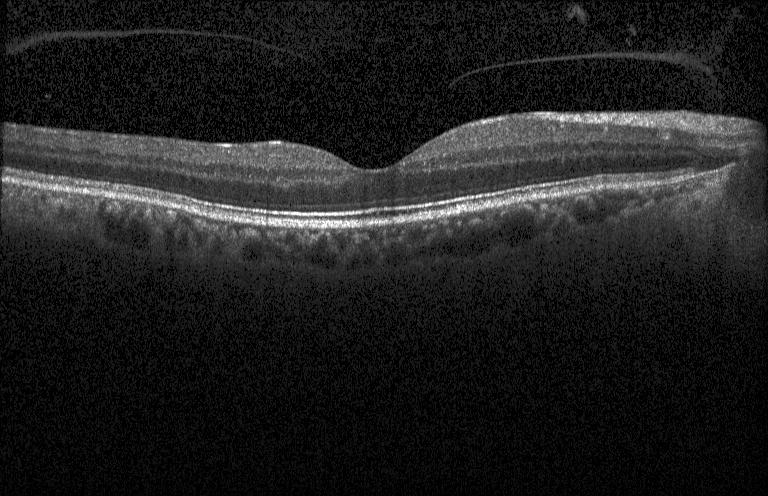
Retinal OCT cross-section showing neither CNV, DME, nor drusen.